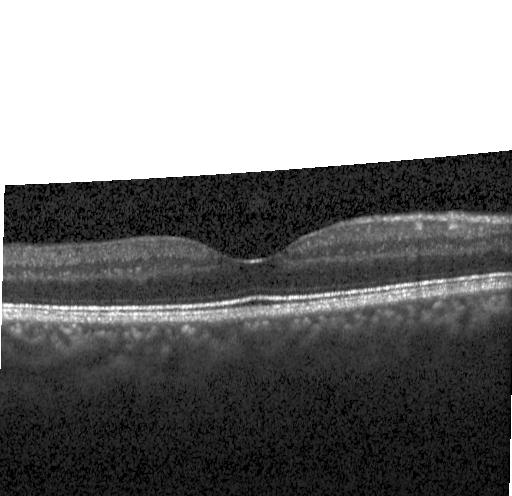

Through the macula; SD-OCT; OCT line scan — Assessment: no choroidal neovascularization, diabetic macular edema, or drusen.